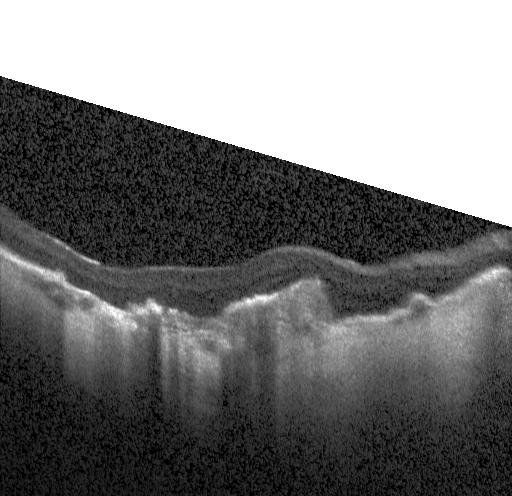 CNV.